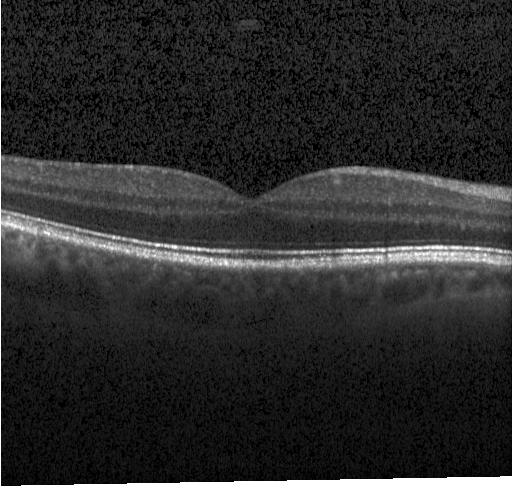

Diagnosis: neither choroidal neovascularization, diabetic macular edema, nor drusen.